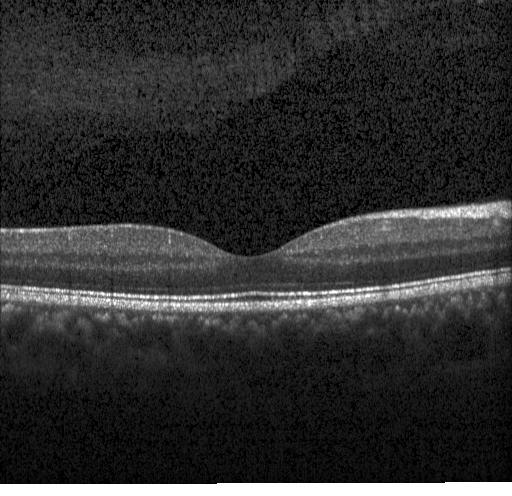 Retinal OCT B-scan
The scan shows no CNV, no DME, and no drusen.